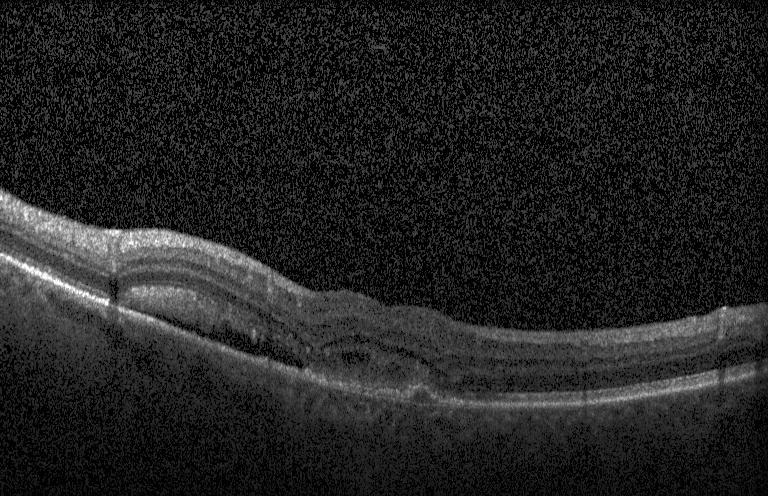
Macular scan, retinal OCT cross-section, SD-OCT, Heidelberg Spectralis
The scan shows a choroidal neovascular membrane.